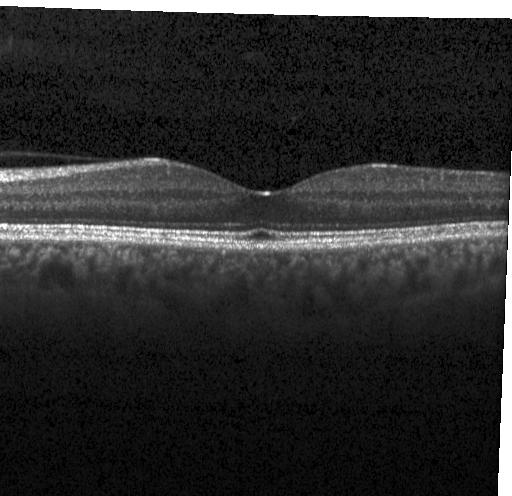

Retinal OCT B-scan. Acquired on a Heidelberg Spectralis. SD-OCT. Horizontal scan through the fovea.
Dx: no evidence of choroidal neovascularization, diabetic macular edema, or drusen.